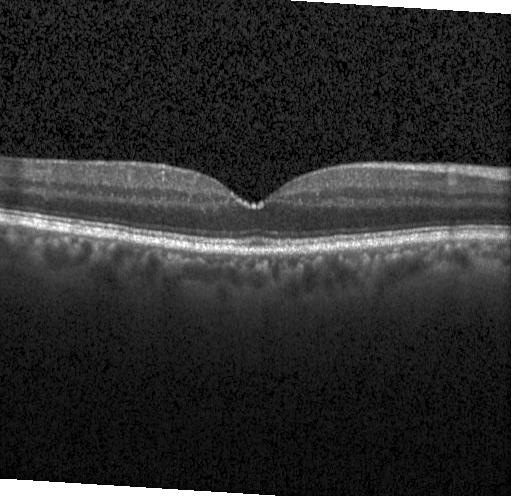
Diagnosis: no choroidal neovascularization, no diabetic macular edema, and no drusen.